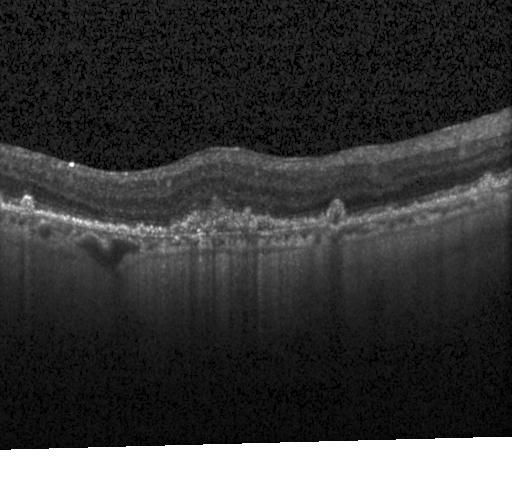
OCT line scan
Finding: a choroidal neovascular membrane.